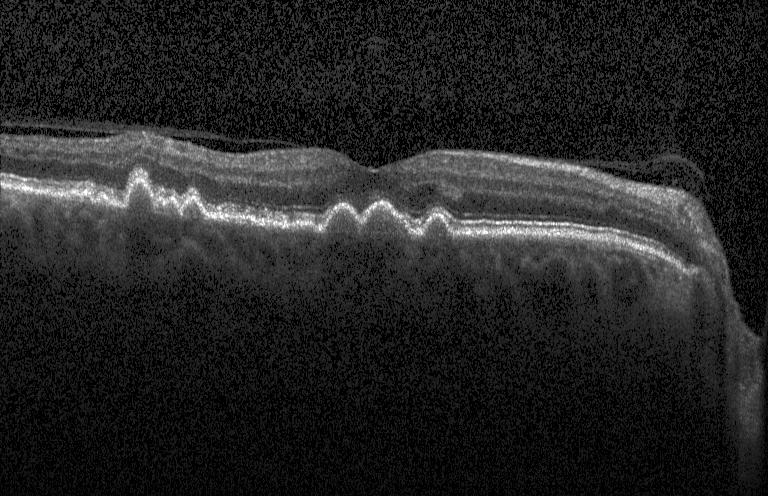

OCT line scan, fovea-centered. Finding: multiple drusen.